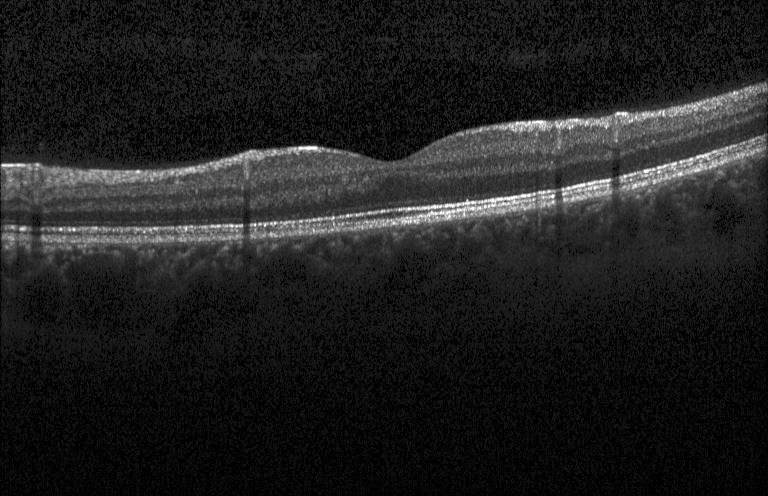

Finding: no evidence of choroidal neovascularization, diabetic macular edema, or drusen.